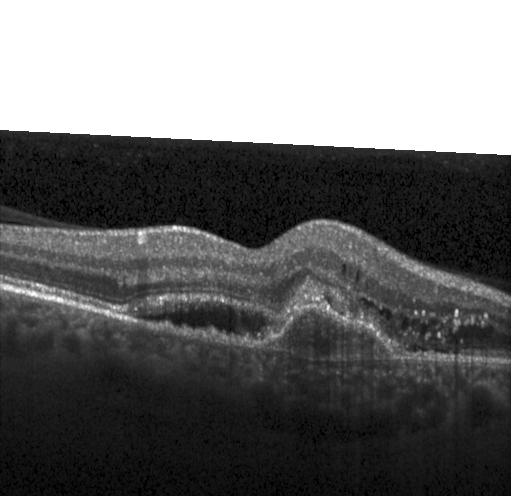 Spectral-domain OCT B-scan: a choroidal neovascular membrane.